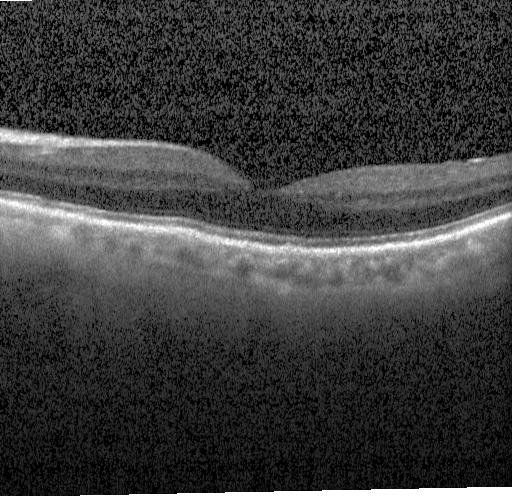
Spectral-domain optical coherence tomography, OCT line scan, acquired on a Heidelberg Spectralis
The scan shows no evidence of CNV, DME, or drusen.